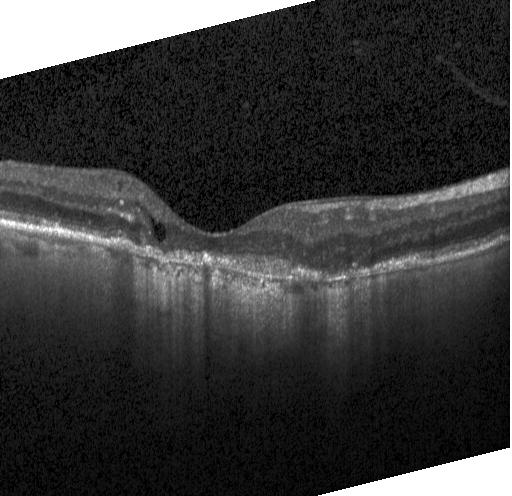 OCT line scan
This B-scan demonstrates choroidal neovascularization.